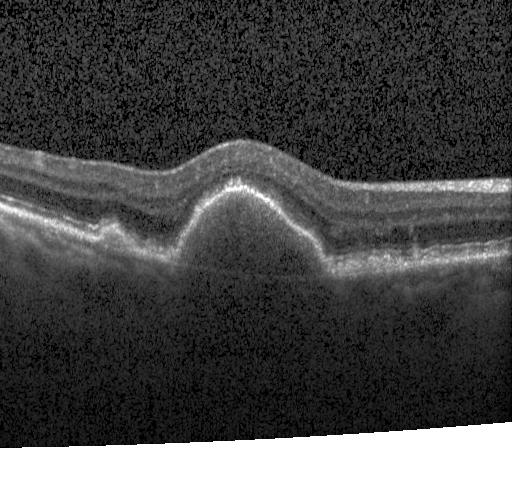 Macular OCT demonstrating choroidal neovascularization.